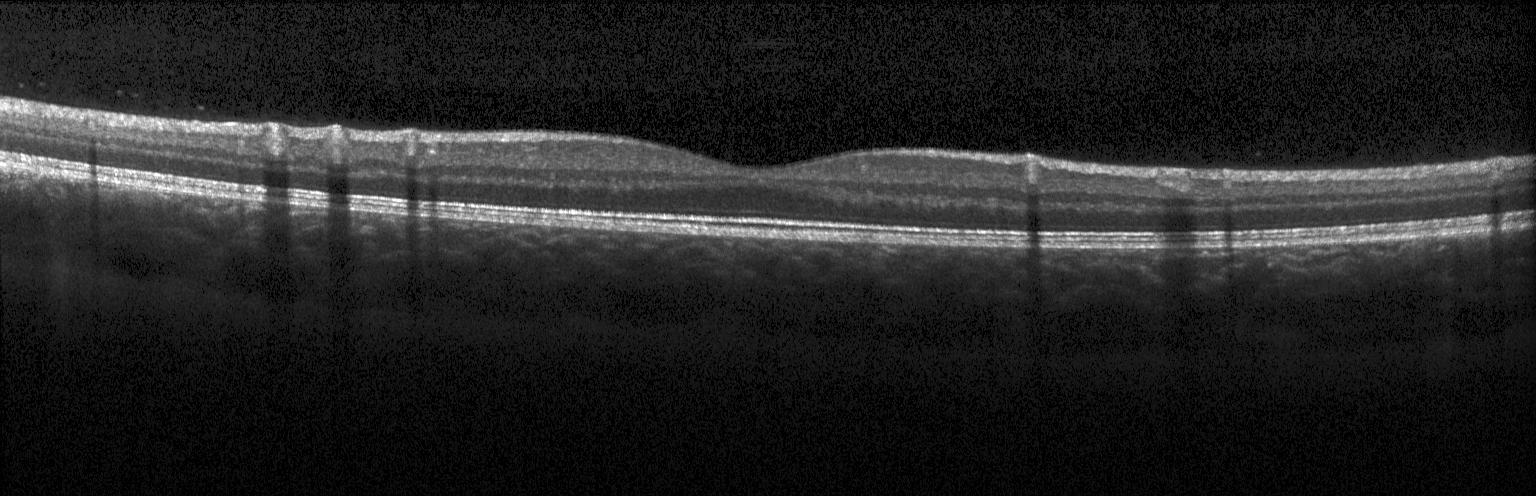
SD-OCT, centered on the fovea, instrument: Heidelberg Spectralis, OCT B-scan.
Dx: no choroidal neovascularization, no diabetic macular edema, and no drusen.